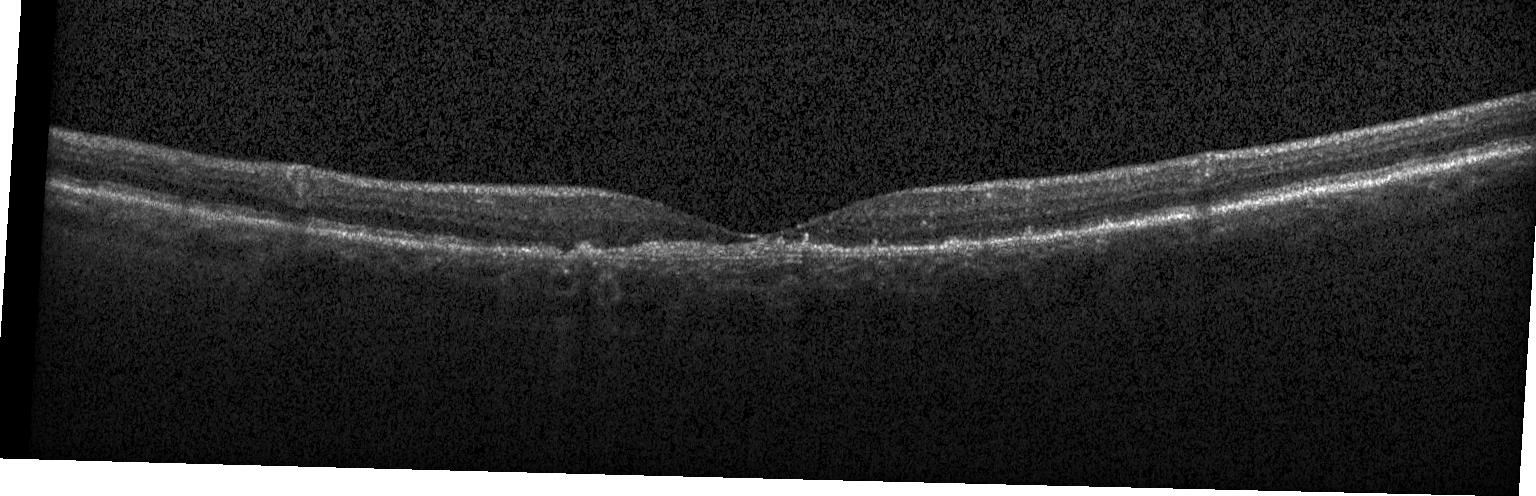

The scan shows choroidal neovascularization.